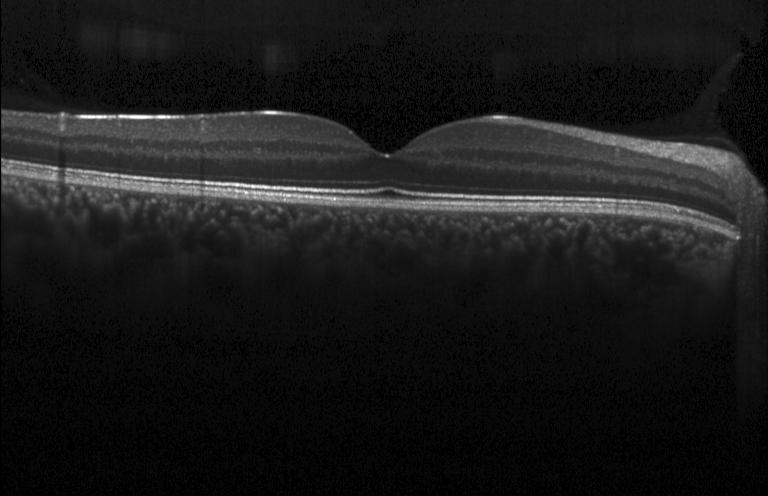 Optical coherence tomography B-scan
Finding: neither choroidal neovascularization, diabetic macular edema, nor drusen.